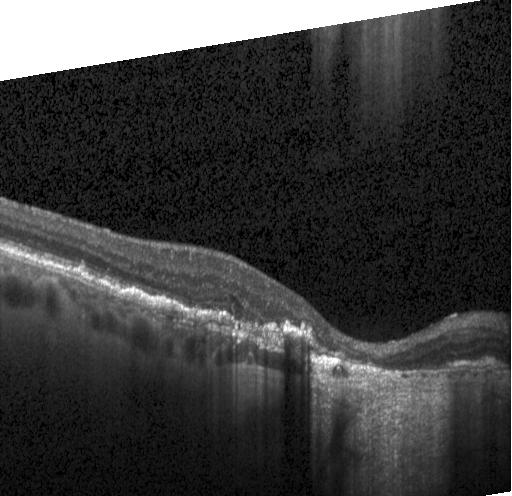 Assessment: a choroidal neovascular membrane.